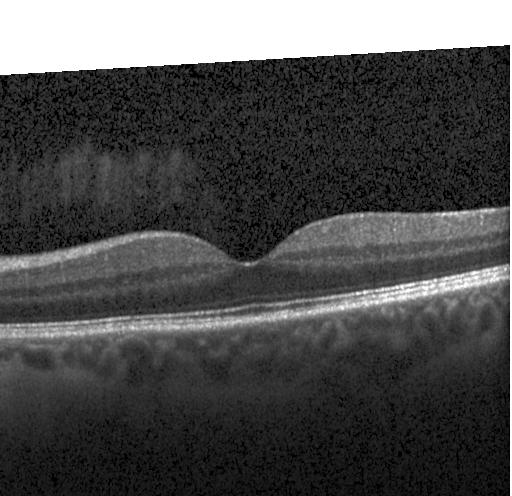
Retinal OCT B-scan
Macular OCT: neither choroidal neovascularization, diabetic macular edema, nor drusen.